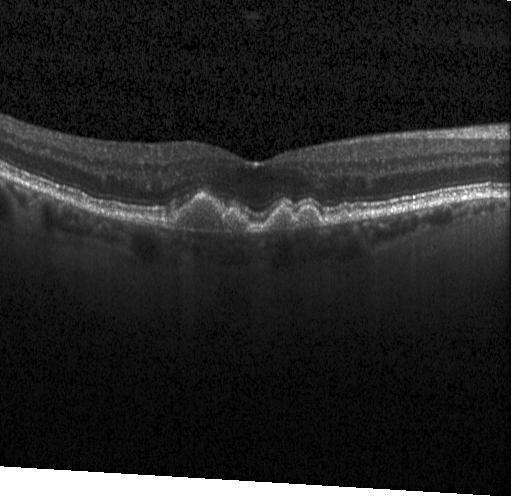 OCT scan showing multiple drusen.